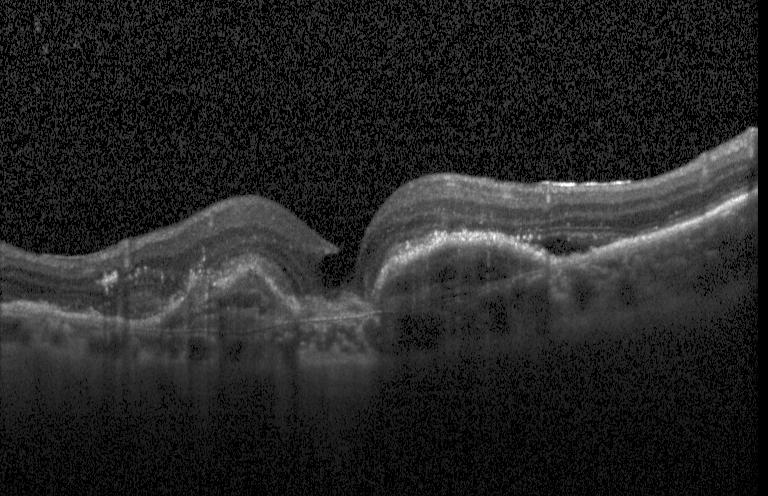
Retinal OCT cross-section; acquired on a Heidelberg Spectralis; horizontal scan through the fovea. Macular OCT: a choroidal neovascular membrane.